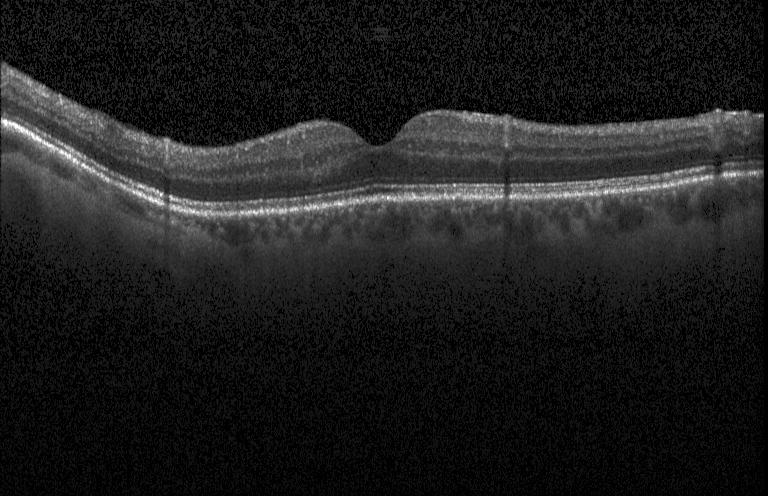
Finding: neither choroidal neovascularization, diabetic macular edema, nor drusen.